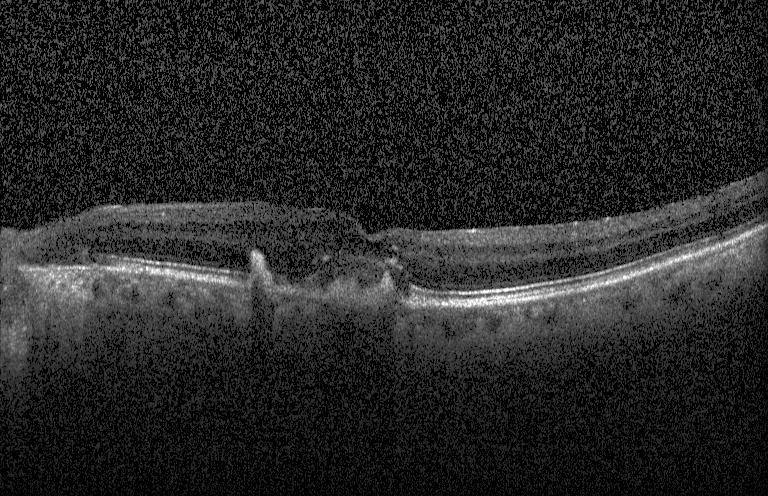

Instrument: Heidelberg Spectralis; retinal OCT cross-section — The scan shows a choroidal neovascular membrane.